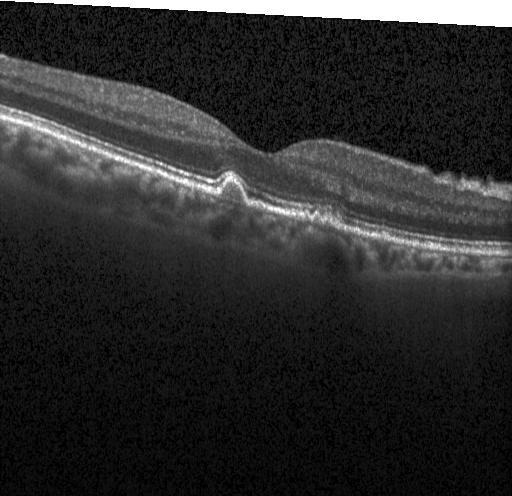 Impression: multiple drusen.